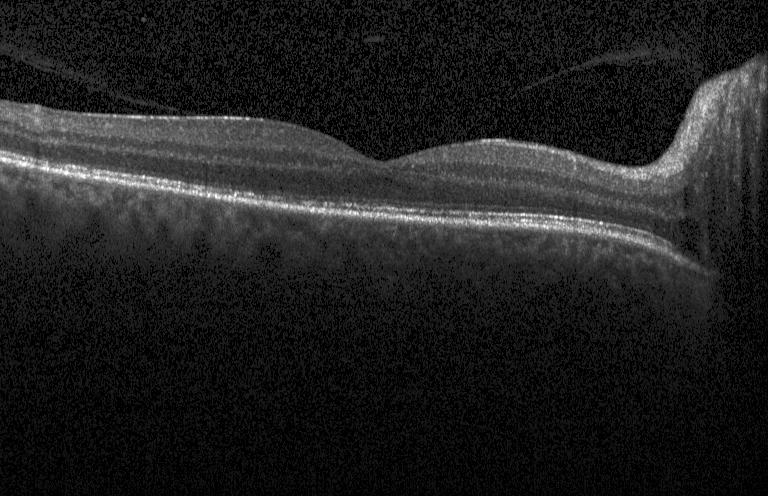
Optical coherence tomography B-scan · spectral-domain optical coherence tomography
Assessment: no evidence of CNV, DME, or drusen.